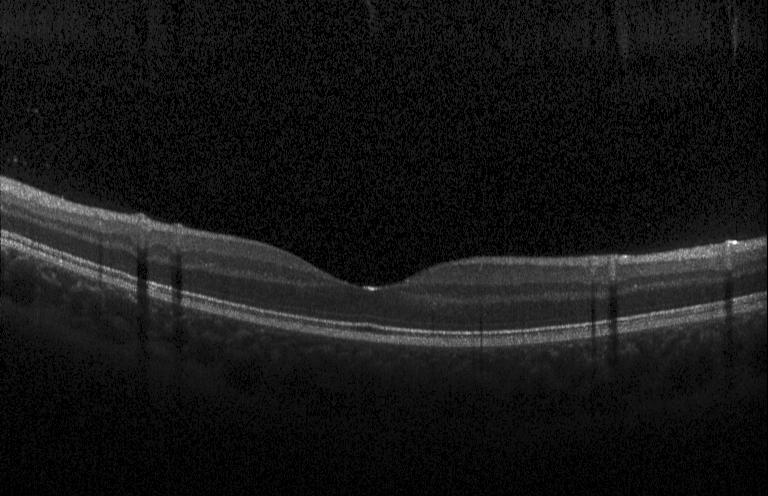
OCT B-scan showing neither choroidal neovascularization, diabetic macular edema, nor drusen.